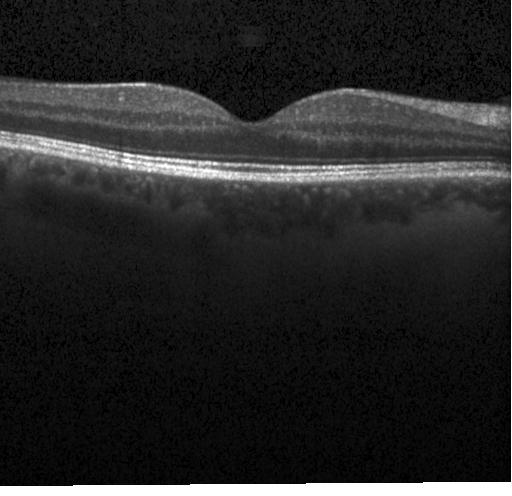 Macular scan · optical coherence tomography scan — Assessment: no evidence of choroidal neovascularization, diabetic macular edema, or drusen.